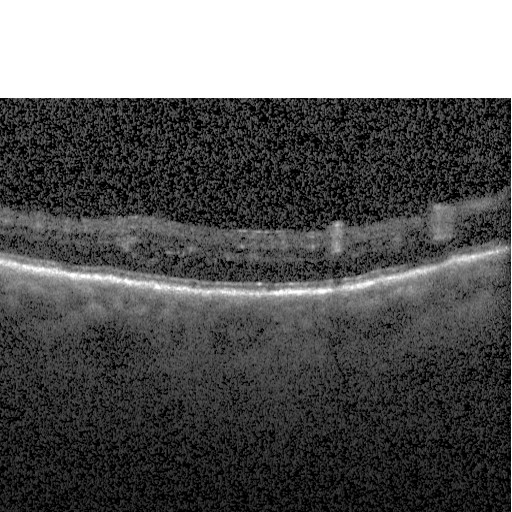
OCT line scan.
Diagnosis: DME.